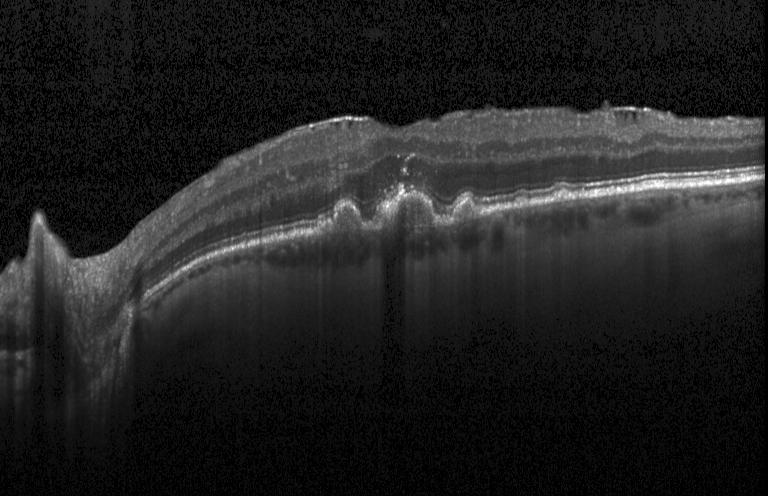
Multiple drusen.